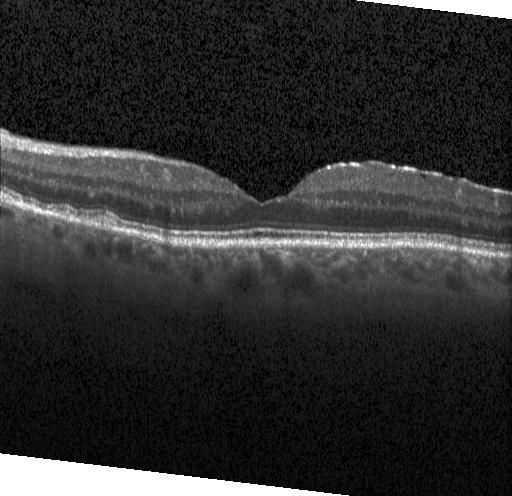 OCT line scan — Finding: multiple drusen.